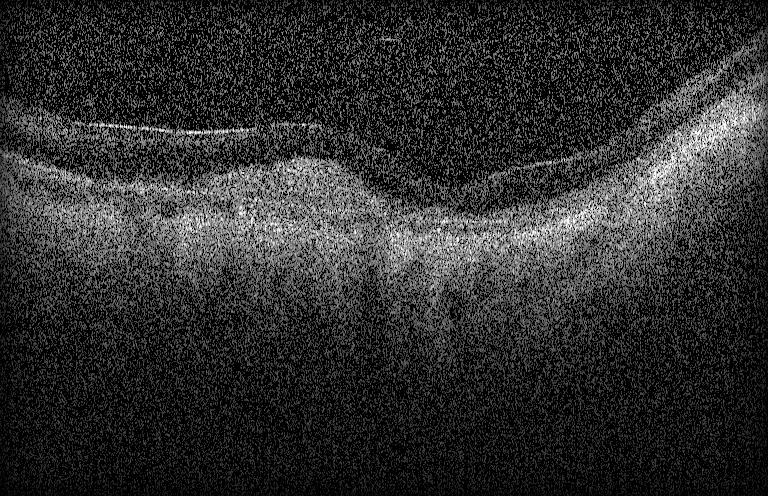

SD-OCT, retinal OCT cross-section, Heidelberg Spectralis OCT system — Diagnosis: CNV.